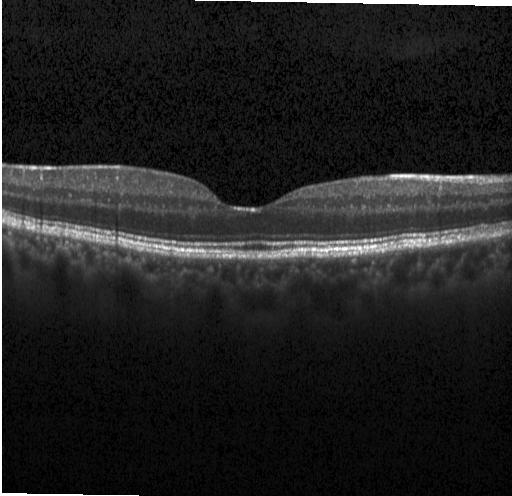
Finding: no choroidal neovascularization, no diabetic macular edema, and no drusen.